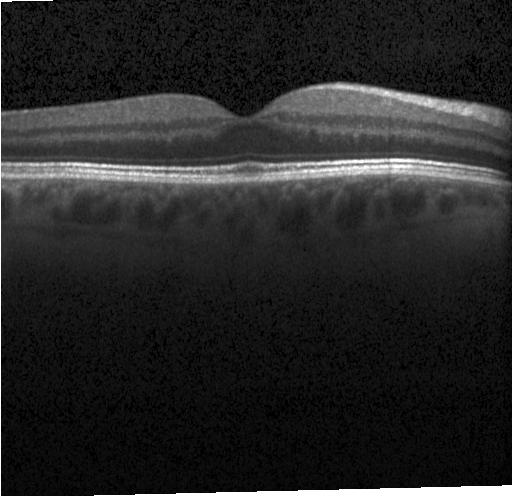

Acquired on a Heidelberg Spectralis. Retinal OCT B-scan — No choroidal neovascularization, diabetic macular edema, or drusen.